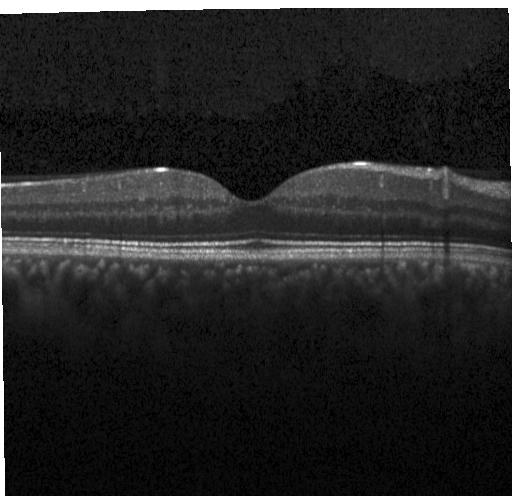

Retinal OCT cross-section, Heidelberg Spectralis, spectral-domain OCT, fovea-centered
Diagnosis: no evidence of CNV, DME, or drusen.